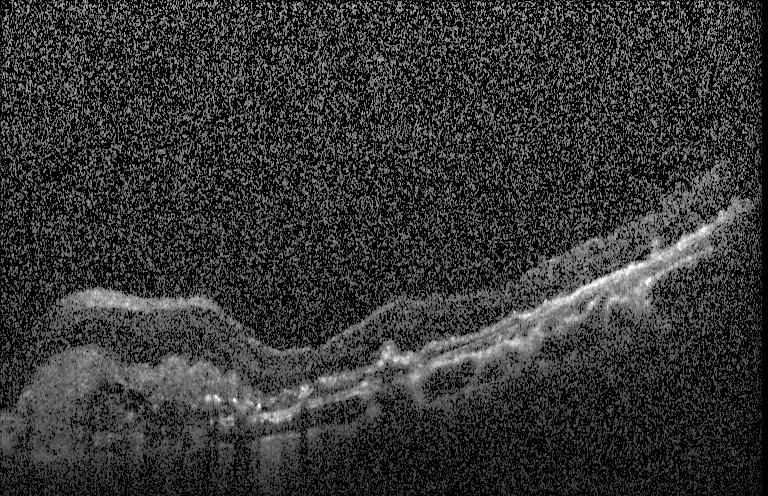 Optical coherence tomography scan
Diagnosis: a choroidal neovascular membrane.